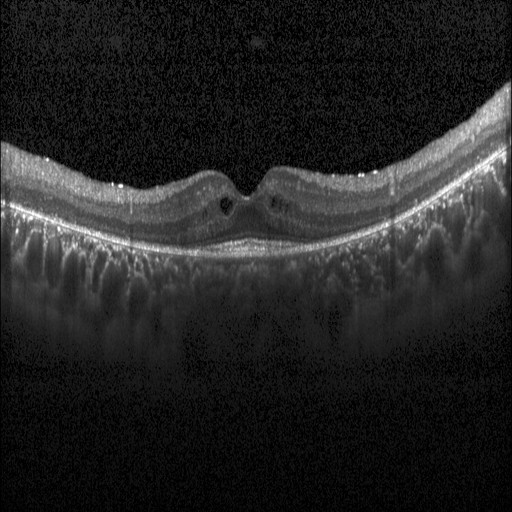 Retinal OCT cross-section; centered on the fovea
Impression: diabetic macular edema (DME).